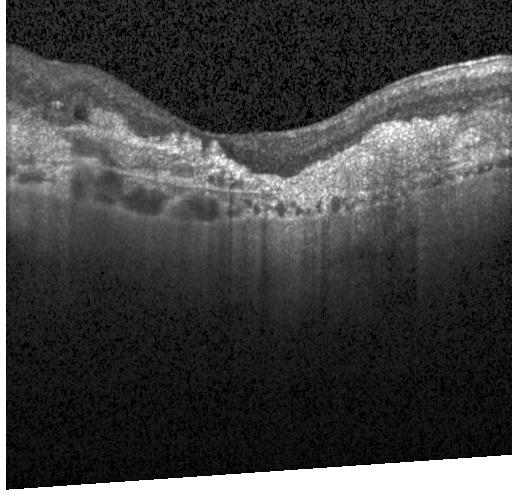

Dx: a choroidal neovascular membrane.